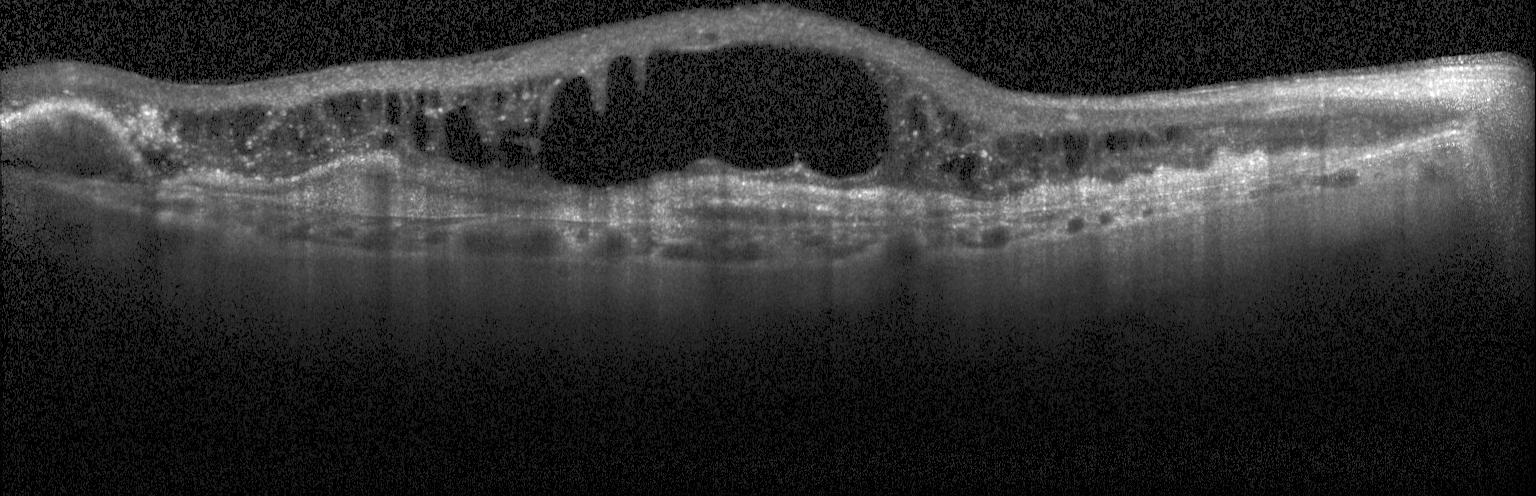 Optical coherence tomography B-scan · fovea-centered.
Diagnosis: choroidal neovascularization (CNV).